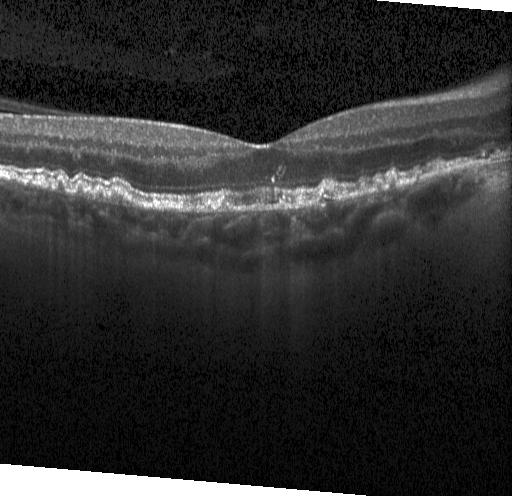
Assessment: a choroidal neovascular membrane.